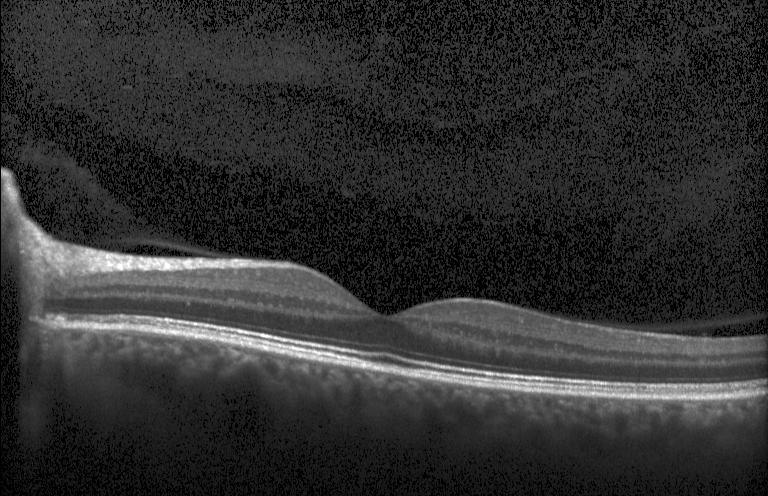

Assessment: no choroidal neovascularization, diabetic macular edema, or drusen.